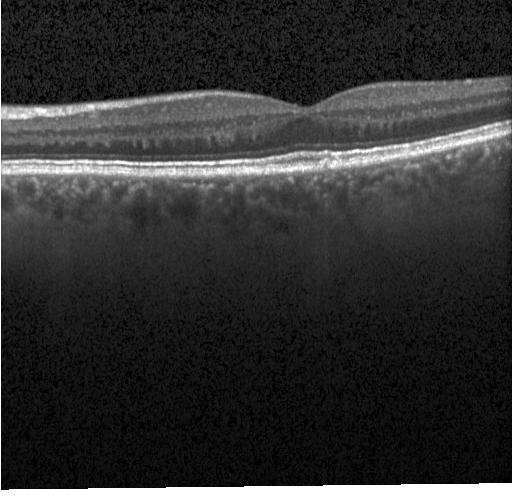
The scan shows no evidence of choroidal neovascularization, diabetic macular edema, or drusen.